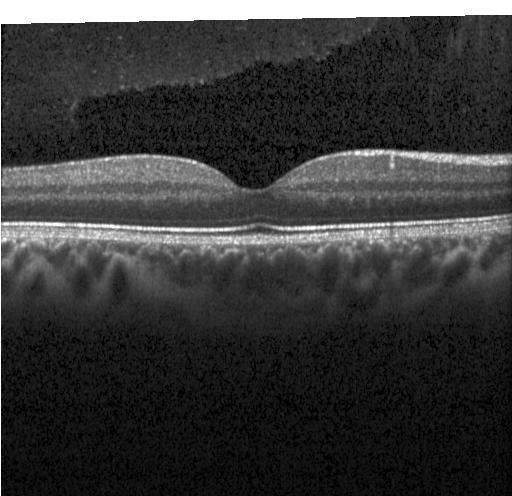 Diagnosis: neither choroidal neovascularization, diabetic macular edema, nor drusen.